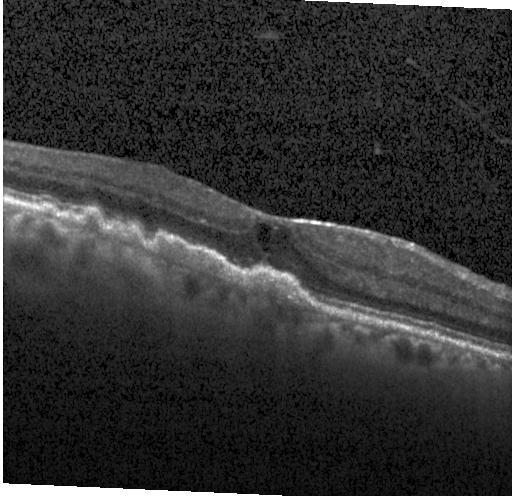 Finding: a choroidal neovascular membrane.